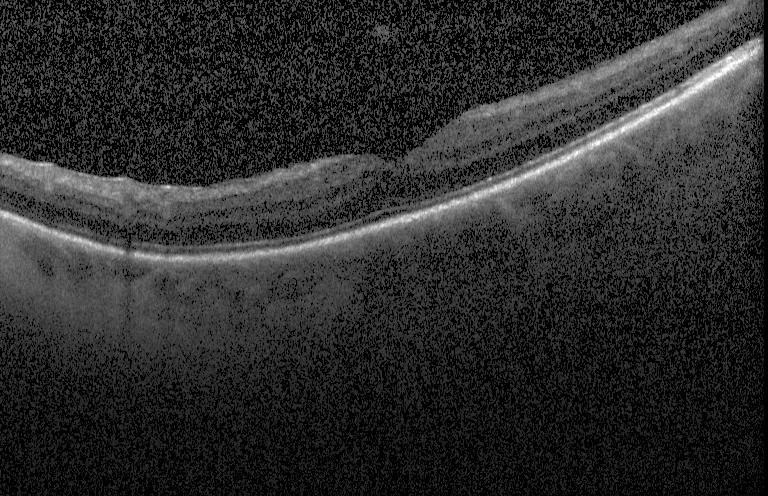
Heidelberg Spectralis · SD-OCT · through the macula · OCT line scan. Impression: no choroidal neovascularization, diabetic macular edema, or drusen.